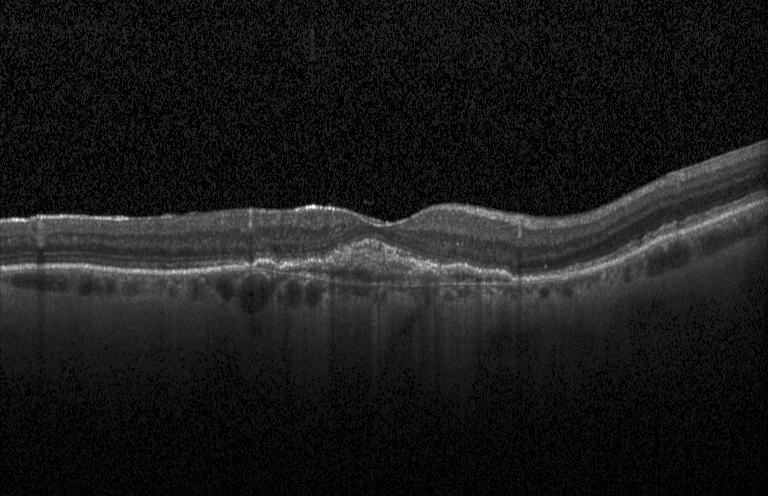
Assessment: a choroidal neovascular membrane.